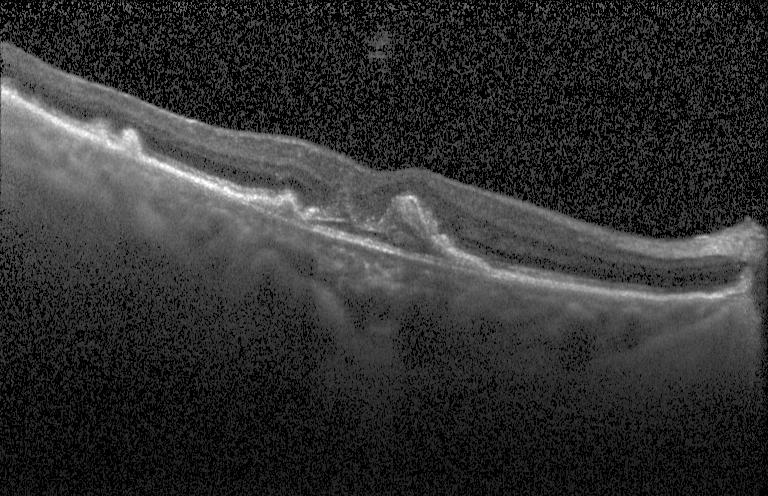 OCT finding: a choroidal neovascular membrane.